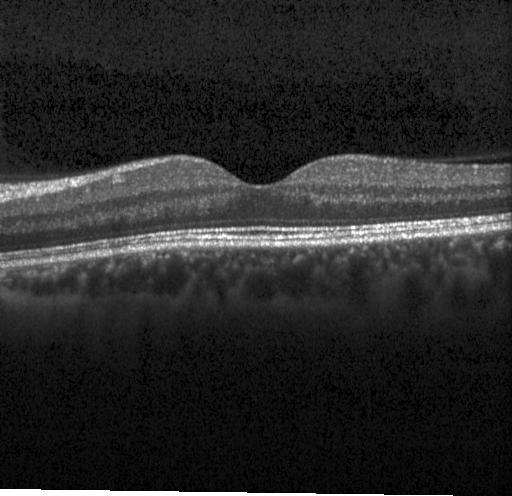

Spectral-domain optical coherence tomography. Optical coherence tomography scan
OCT finding: neither choroidal neovascularization, diabetic macular edema, nor drusen.